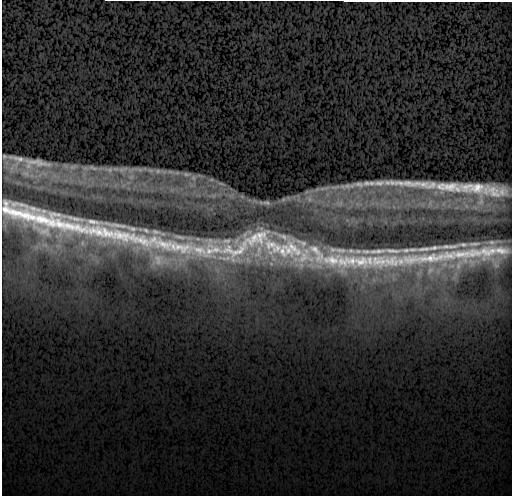 Diagnosis: drusen.